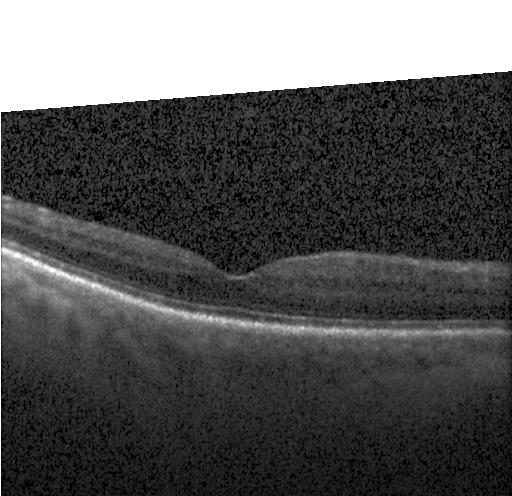 Centered on the fovea; optical coherence tomography scan; spectral-domain optical coherence tomography
This B-scan demonstrates neither choroidal neovascularization, diabetic macular edema, nor drusen.